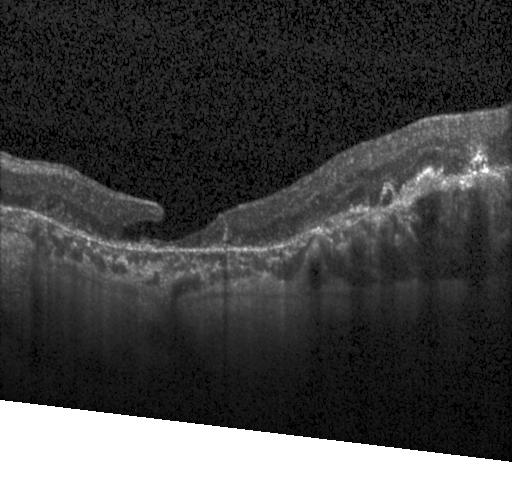 OCT B-scan showing CNV.